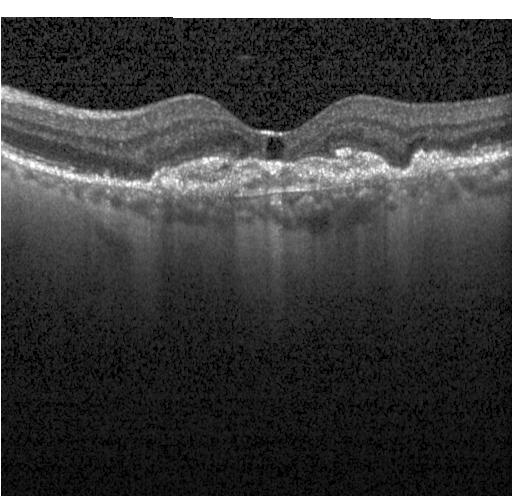 Spectral-domain OCT. Heidelberg Spectralis. Centered on the fovea. Retinal OCT cross-section. Finding: a choroidal neovascular membrane.